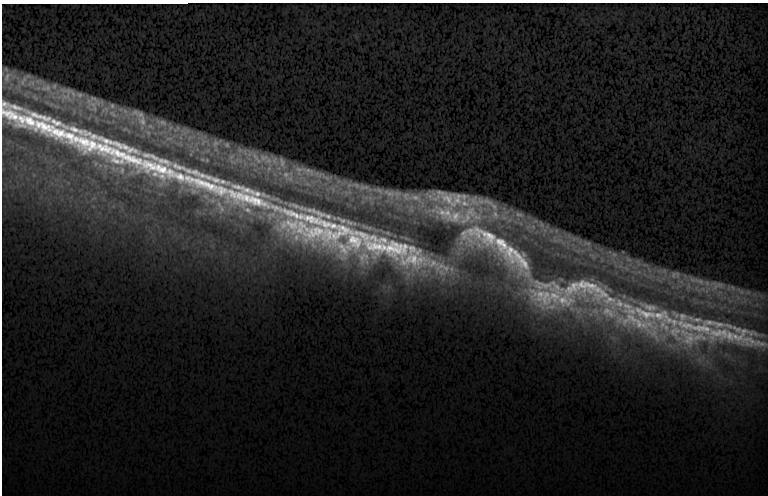

Optical coherence tomography B-scan, fovea-centered, acquired on a Heidelberg Spectralis, spectral-domain OCT.
Impression: choroidal neovascularization (CNV).